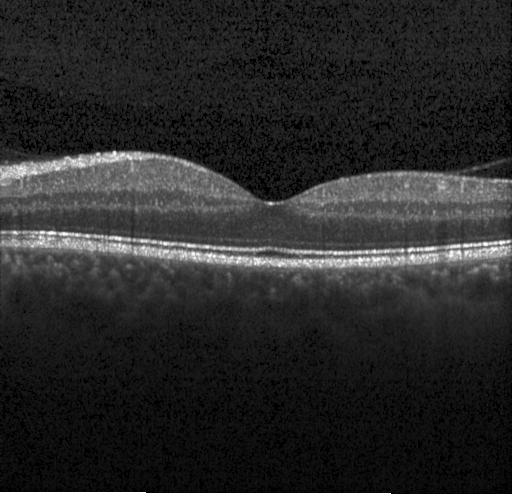

Optical coherence tomography B-scan. Macular OCT: no choroidal neovascularization, diabetic macular edema, or drusen.